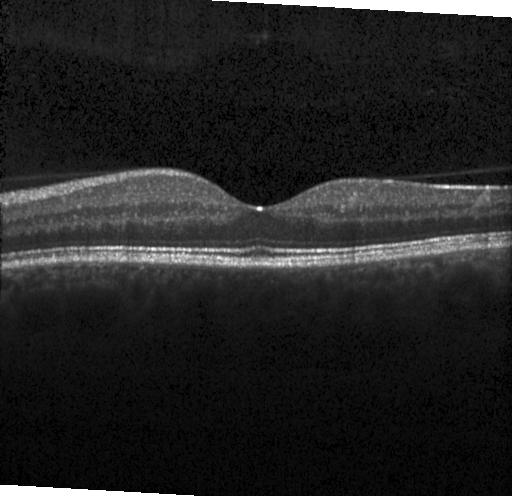 Dx: no choroidal neovascularization, diabetic macular edema, or drusen.